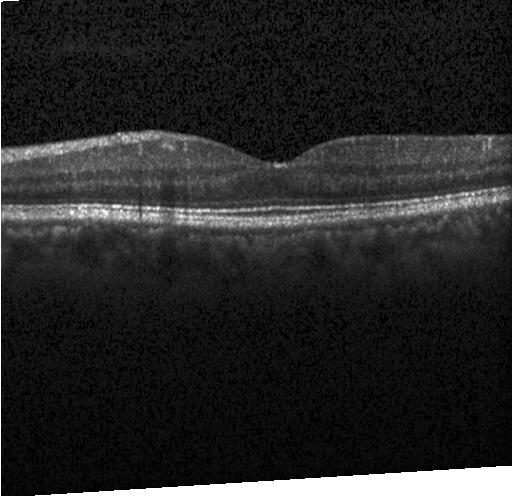

Retinal OCT B-scan; through the macula. Dx: no evidence of choroidal neovascularization, diabetic macular edema, or drusen.